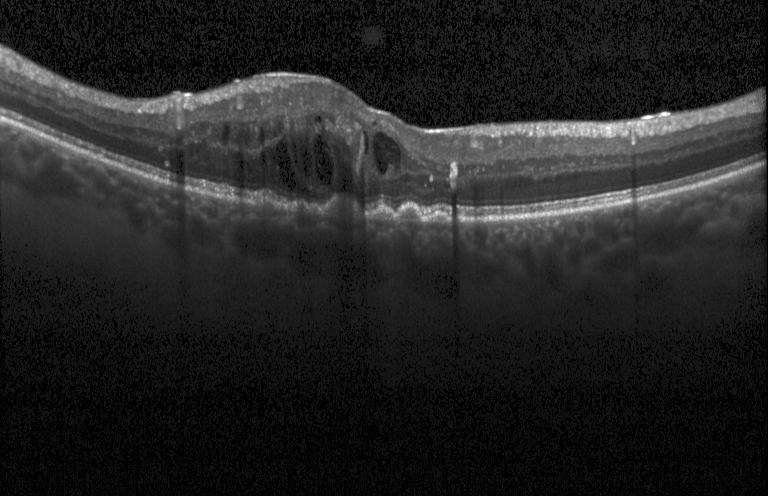
Through the macula, OCT B-scan. OCT finding: DME.